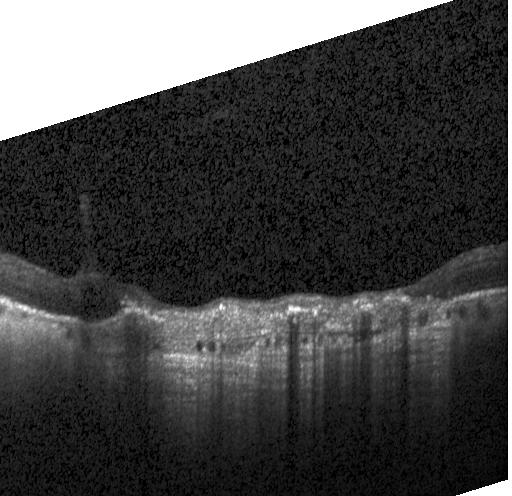 Centered on the fovea · optical coherence tomography B-scan · spectral-domain OCT. Dx: a choroidal neovascular membrane.